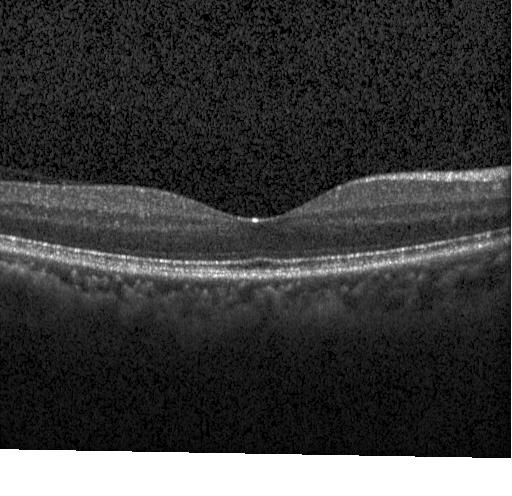
OCT B-scan showing no evidence of CNV, DME, or drusen.